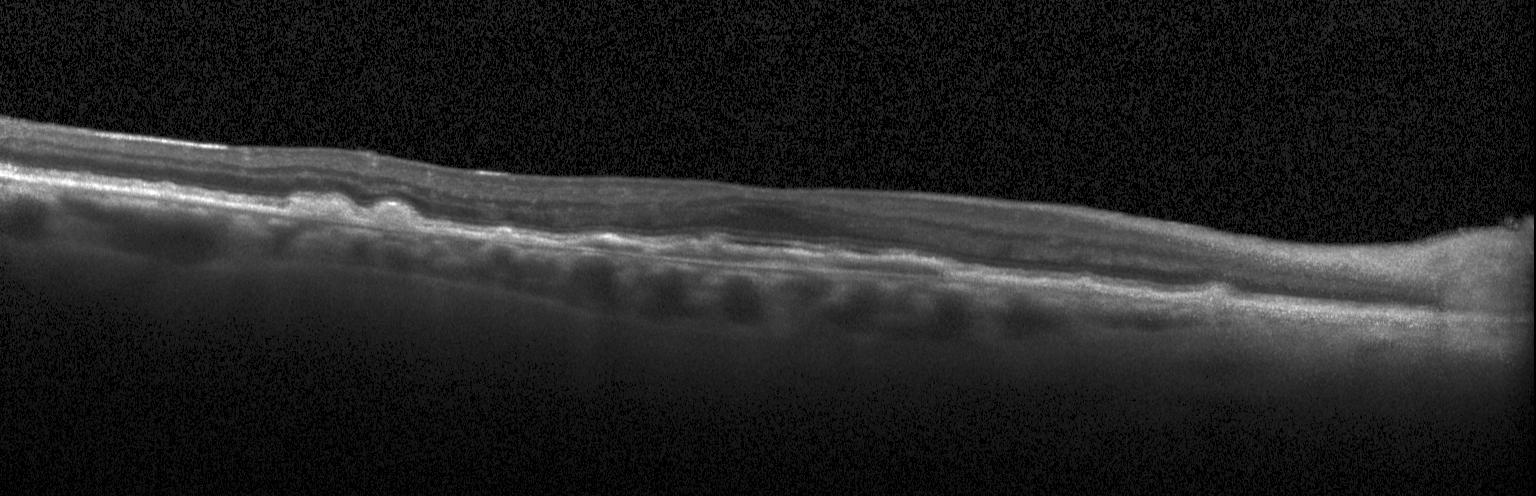 SD-OCT, macular scan, retinal OCT B-scan, Heidelberg Spectralis
Dx: choroidal neovascularization (CNV).